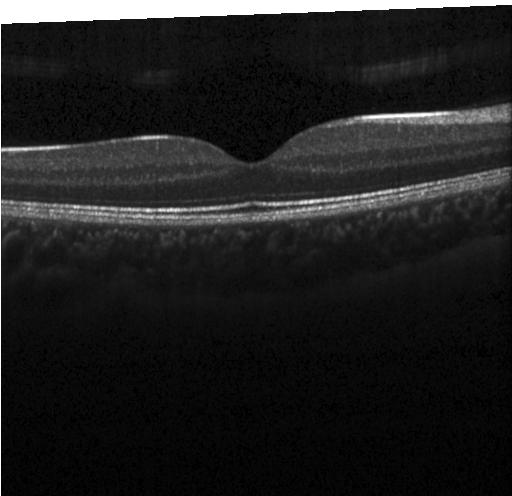
Horizontal scan through the fovea · OCT line scan · spectral-domain OCT
OCT finding: neither CNV, DME, nor drusen.